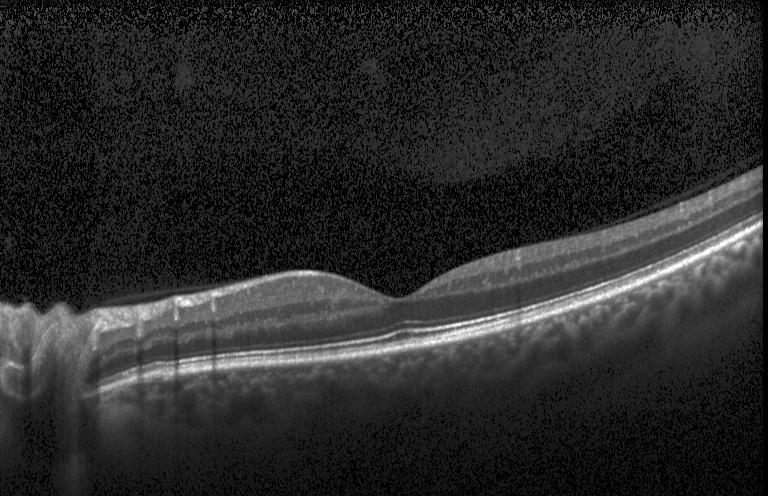 Retinal OCT cross-section — Finding: no choroidal neovascularization, diabetic macular edema, or drusen.